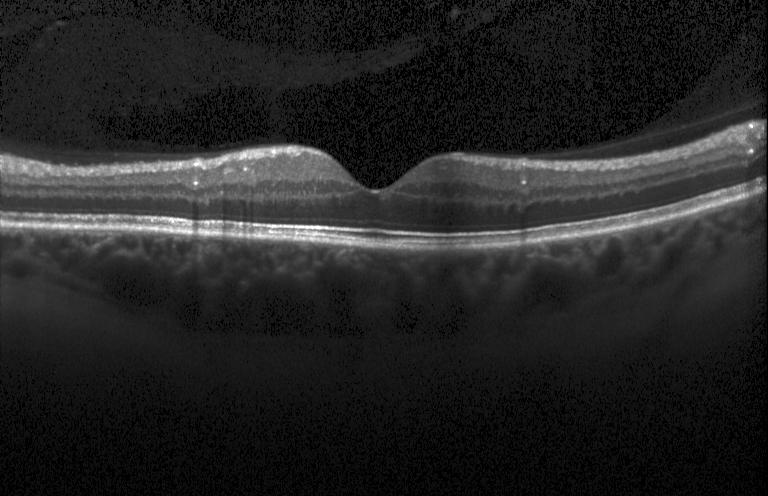 Heidelberg Spectralis OCT system; OCT B-scan; SD-OCT — Assessment: no evidence of choroidal neovascularization, diabetic macular edema, or drusen.